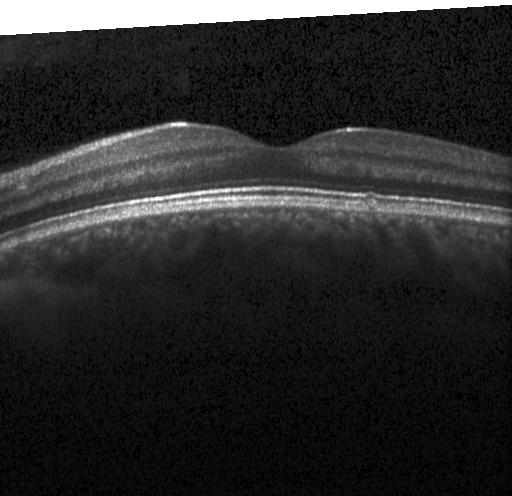

Retinal OCT B-scan. Assessment: no evidence of CNV, DME, or drusen.